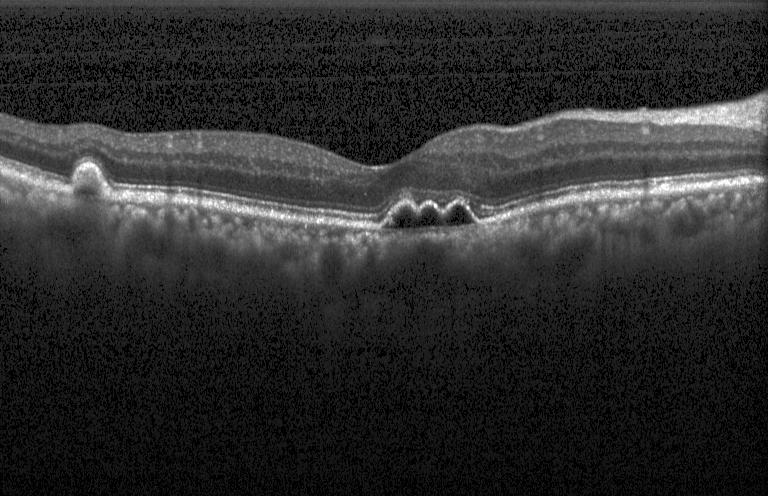 Impression: choroidal neovascularization (CNV).